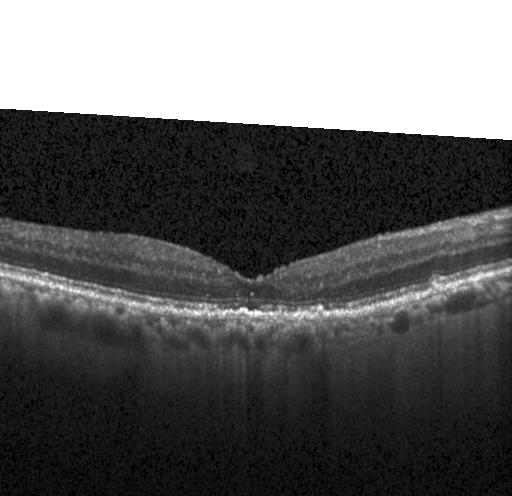

Acquired on a Heidelberg Spectralis; optical coherence tomography B-scan; SD-OCT
Finding: sub-RPE drusenoid deposits.